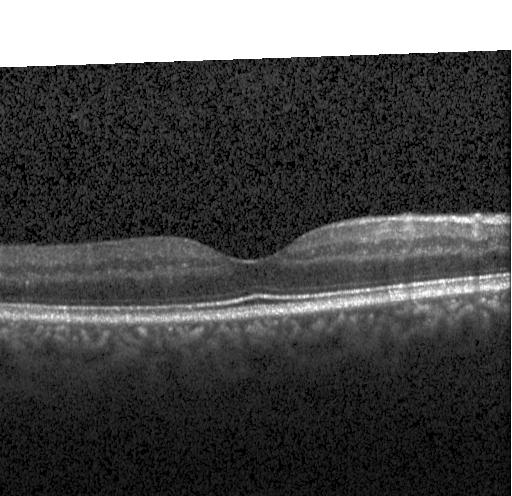 Heidelberg Spectralis; optical coherence tomography B-scan — Diagnosis: neither CNV, DME, nor drusen.